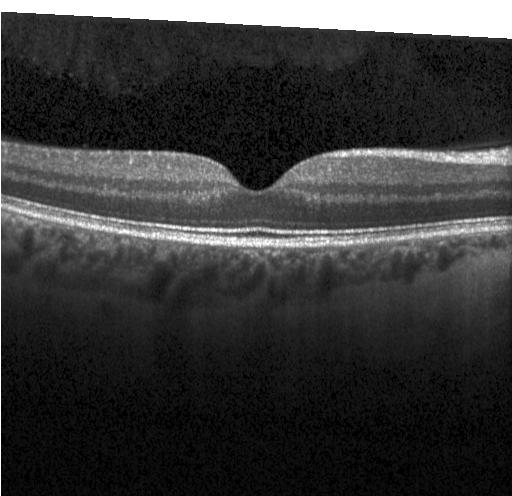

This B-scan demonstrates no choroidal neovascularization, diabetic macular edema, or drusen.